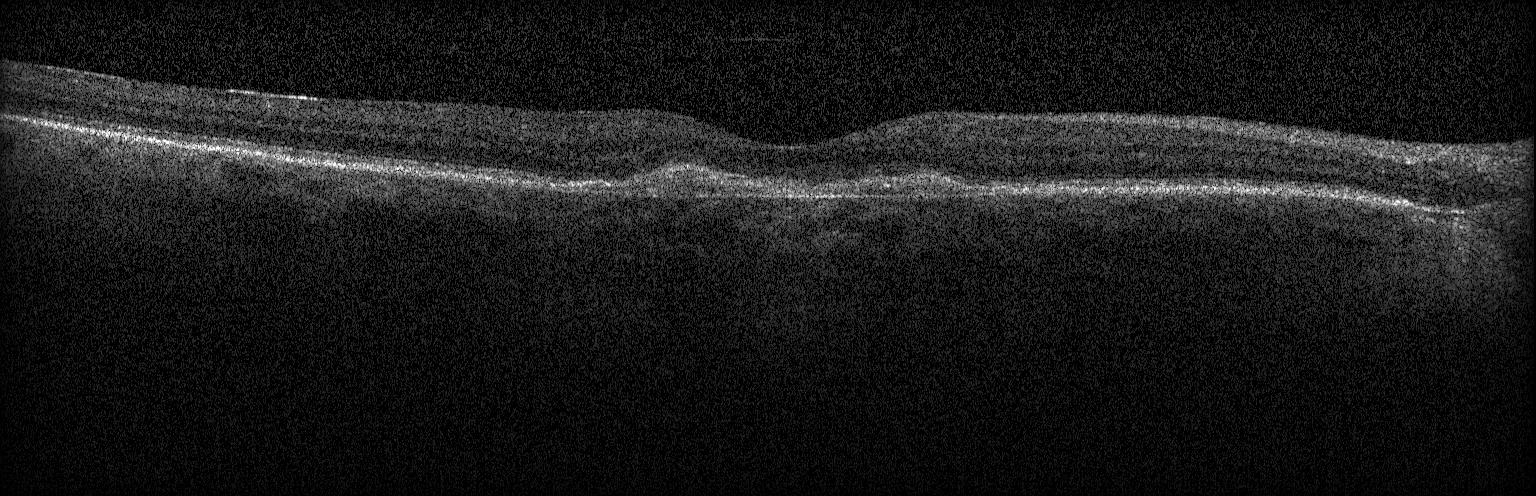
Spectral-domain OCT · horizontal scan through the fovea · OCT B-scan · instrument: Heidelberg Spectralis — Assessment: choroidal neovascularization (CNV).